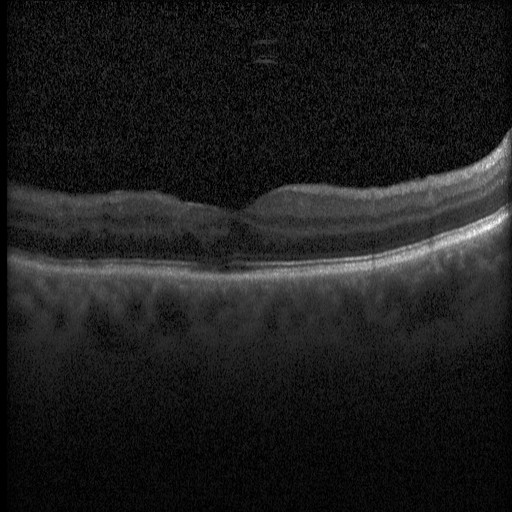

OCT scan showing diabetic macular edema.